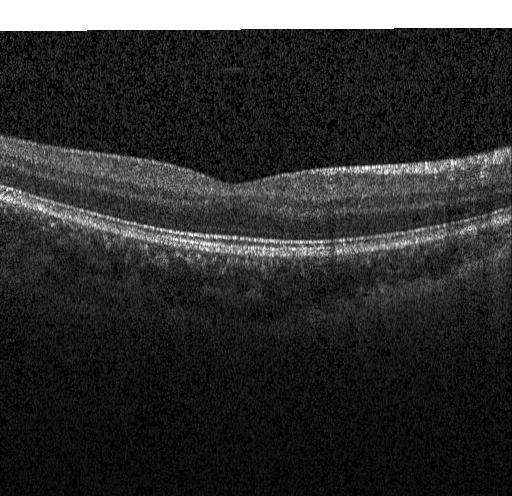
OCT finding: no choroidal neovascularization, no diabetic macular edema, and no drusen.